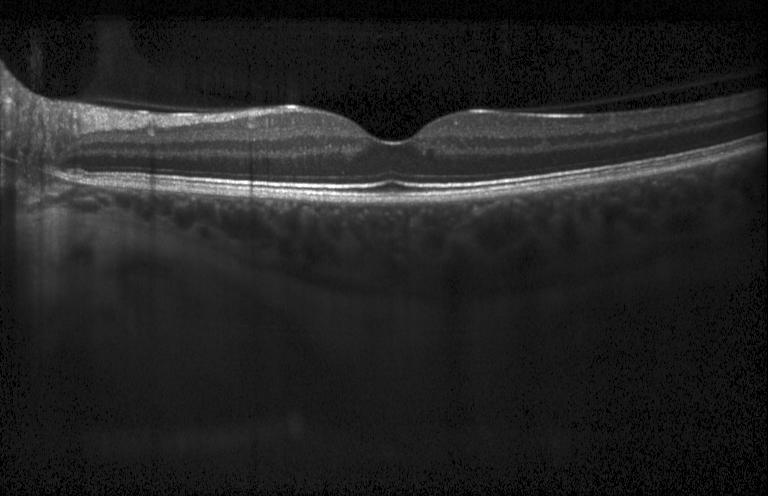

Diagnosis: no choroidal neovascularization, diabetic macular edema, or drusen.